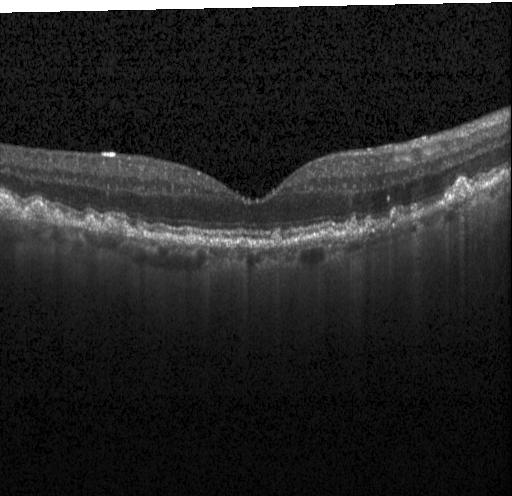
Spectral-domain optical coherence tomography · optical coherence tomography scan — Impression: drusen.